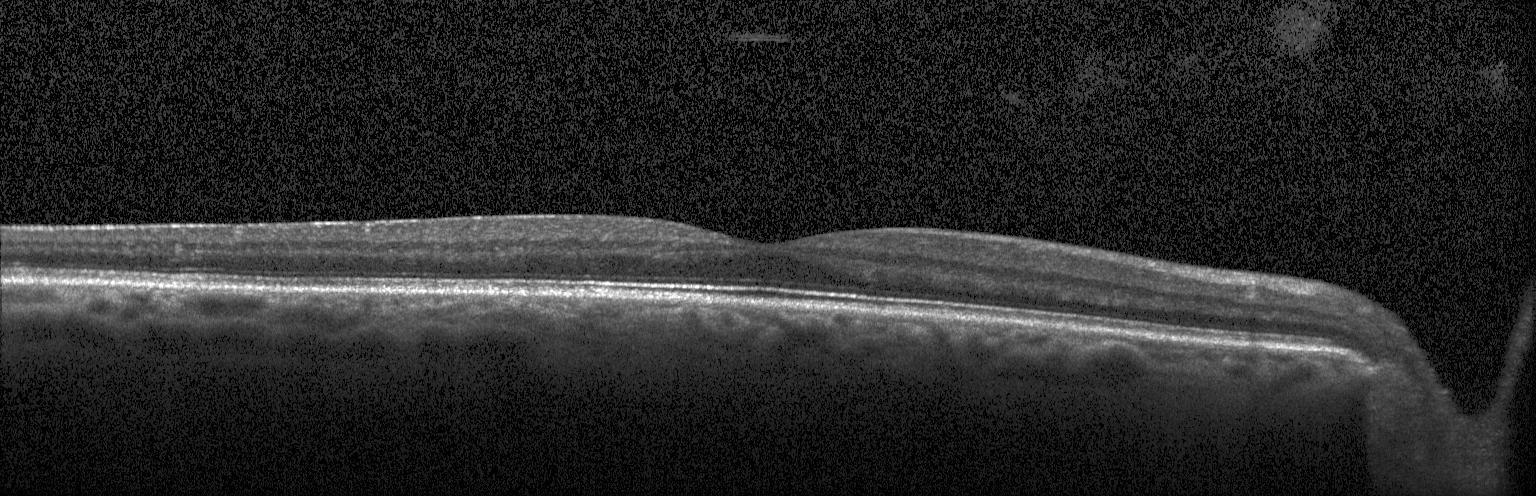
Centered on the fovea, retinal OCT B-scan — Assessment: no choroidal neovascularization, diabetic macular edema, or drusen.